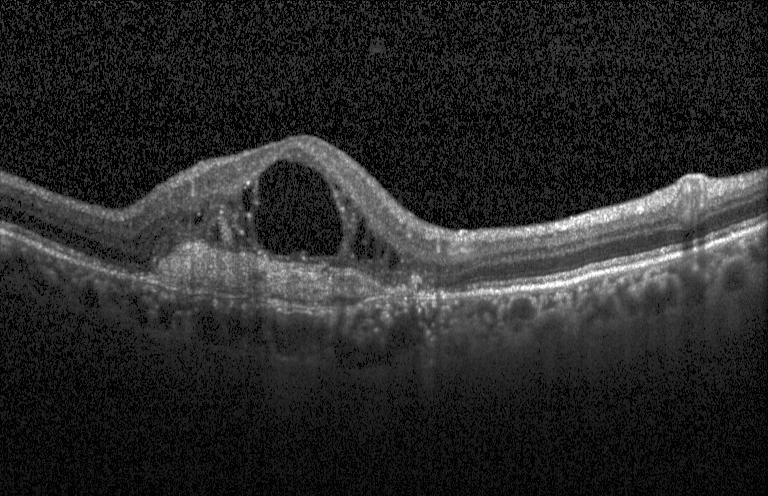 OCT line scan, spectral-domain OCT
Diagnosis: a choroidal neovascular membrane.